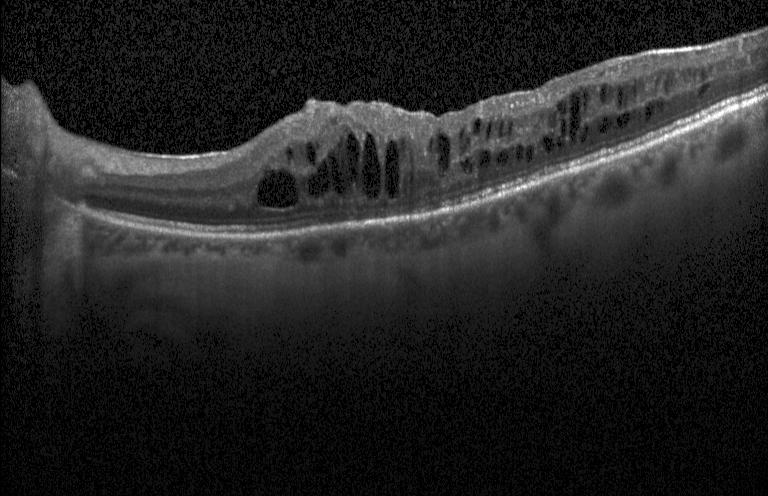

Optical coherence tomography scan. Heidelberg Spectralis — Diagnosis: DME.